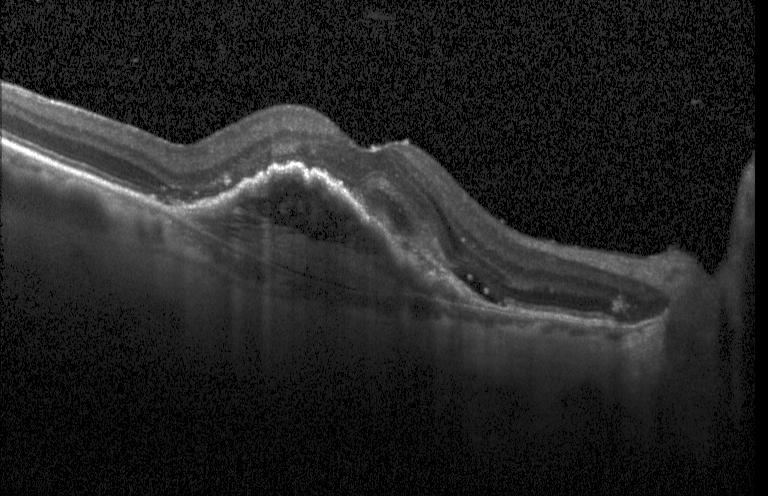
Optical coherence tomography scan. Assessment: a choroidal neovascular membrane.